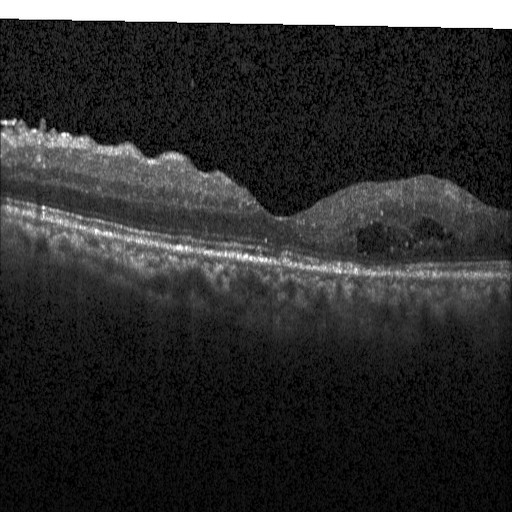 Optical coherence tomography scan. Impression: diabetic macular edema.